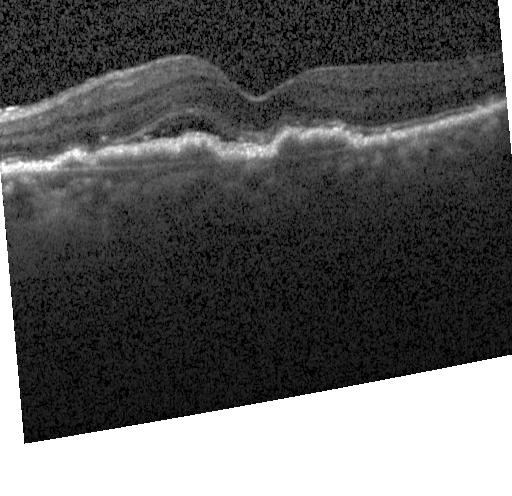
Spectral-domain optical coherence tomography; OCT B-scan; fovea-centered; acquired on a Heidelberg Spectralis
Assessment: a choroidal neovascular membrane.